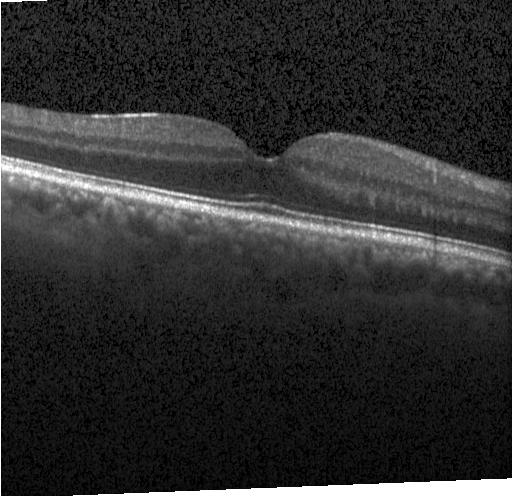
The scan shows no evidence of choroidal neovascularization, diabetic macular edema, or drusen.